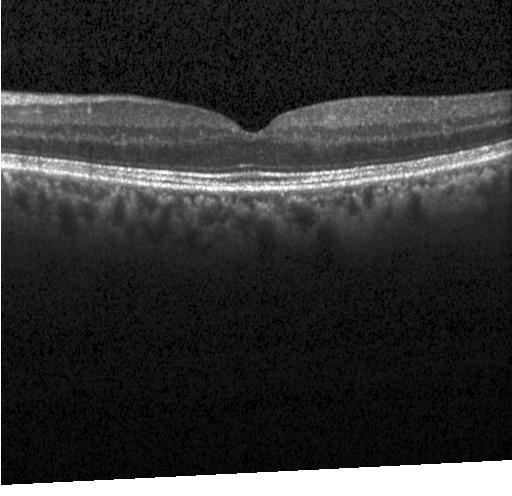
Impression: no choroidal neovascularization, no diabetic macular edema, and no drusen.